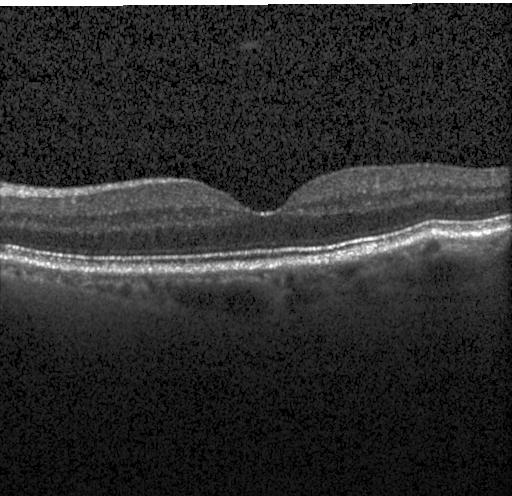
Heidelberg Spectralis OCT system, spectral-domain OCT, through the macula, optical coherence tomography scan. Diagnosis: no choroidal neovascularization, diabetic macular edema, or drusen.